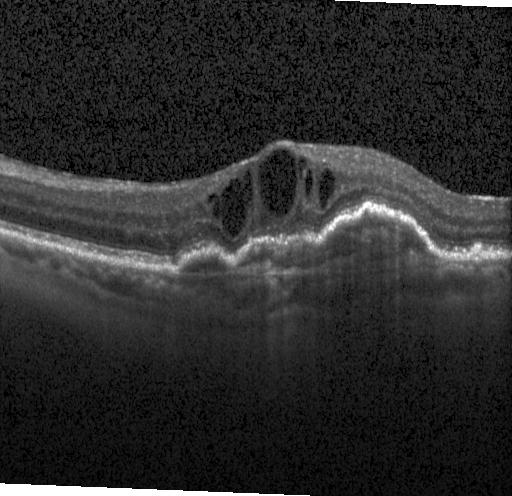
Optical coherence tomography B-scan
Diagnosis: a choroidal neovascular membrane.